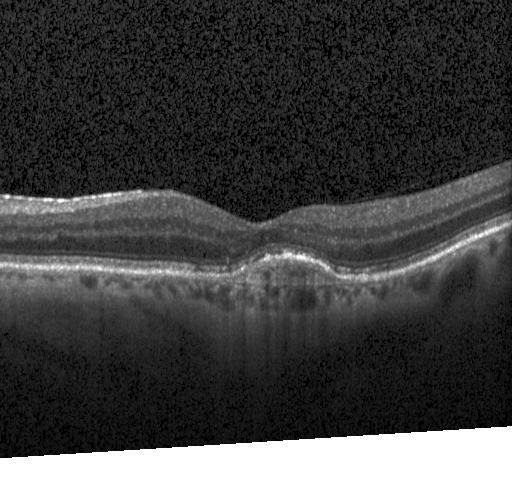 Optical coherence tomography scan, SD-OCT, fovea-centered
Impression: CNV.